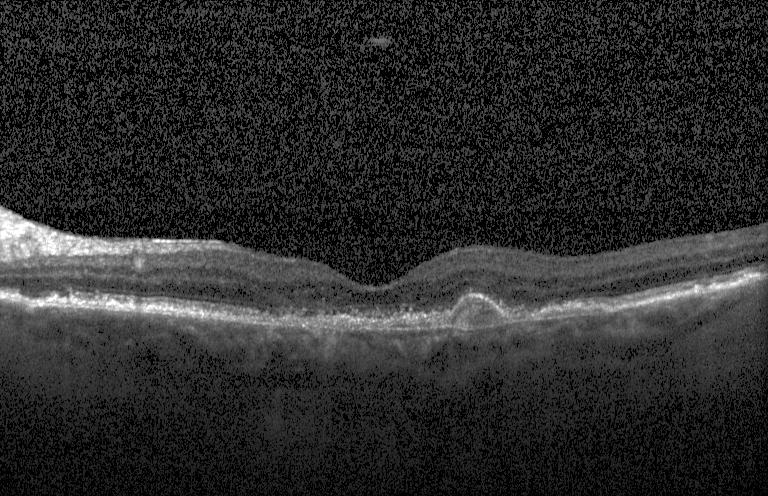

This B-scan demonstrates a choroidal neovascular membrane.